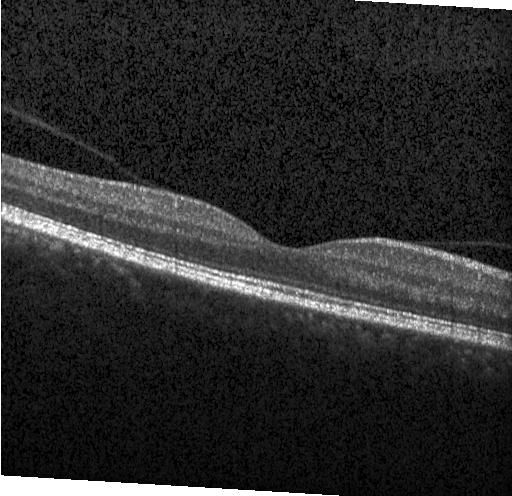

Optical coherence tomography scan — Impression: neither CNV, DME, nor drusen.